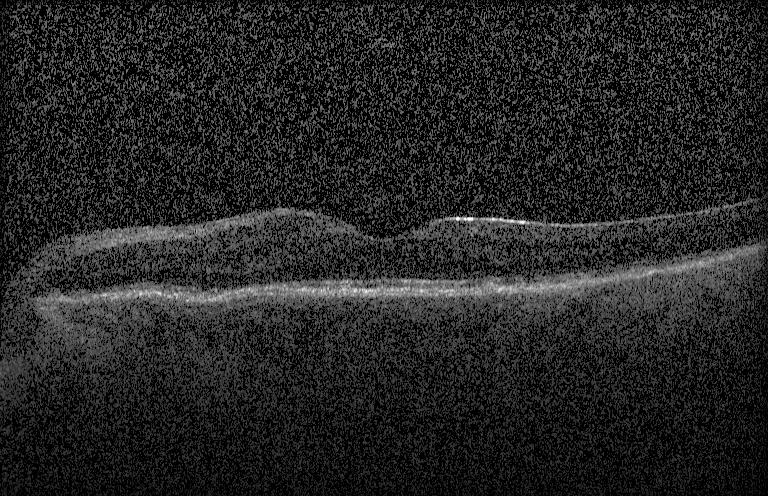
Optical coherence tomography B-scan; SD-OCT; horizontal scan through the fovea; instrument: Heidelberg Spectralis — This B-scan demonstrates no choroidal neovascularization, no diabetic macular edema, and no drusen.